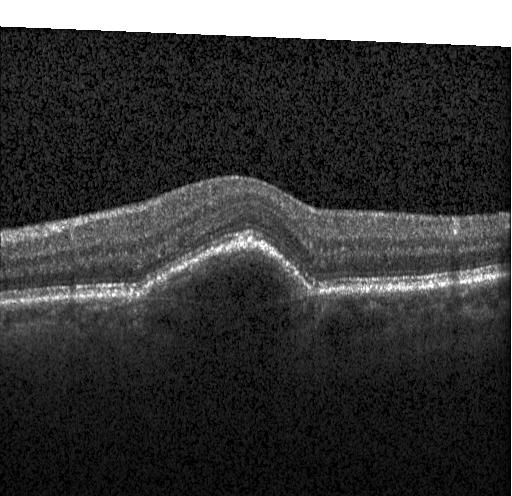
Fovea-centered; retinal OCT B-scan; spectral-domain OCT.
Macular OCT: choroidal neovascularization (CNV).